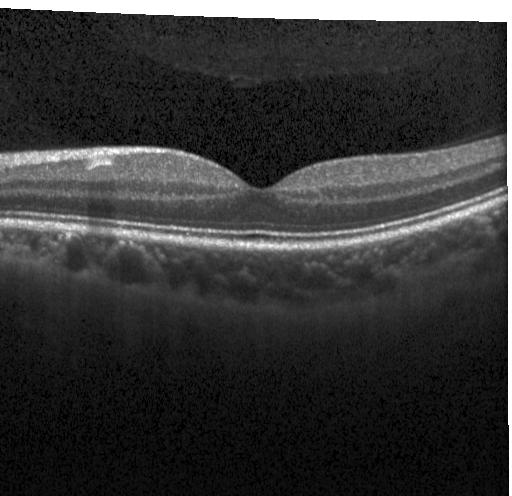
Spectral-domain optical coherence tomography · OCT line scan. Impression: no choroidal neovascularization, diabetic macular edema, or drusen.